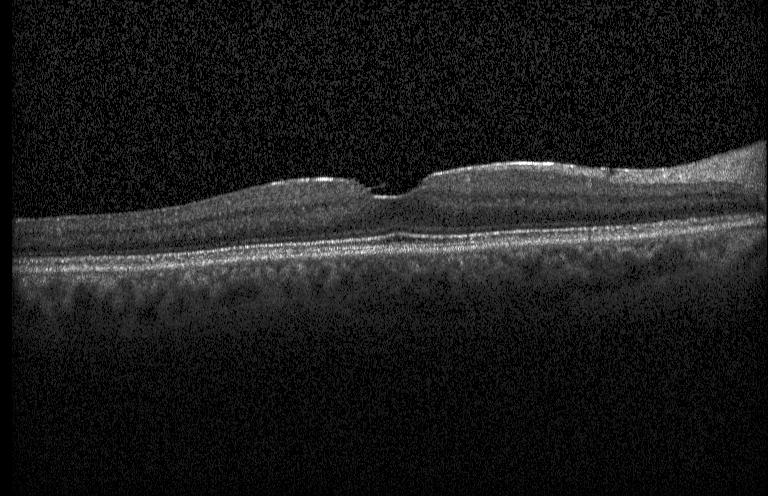
OCT B-scan · Heidelberg Spectralis OCT system · through the macula — This B-scan demonstrates no evidence of choroidal neovascularization, diabetic macular edema, or drusen.